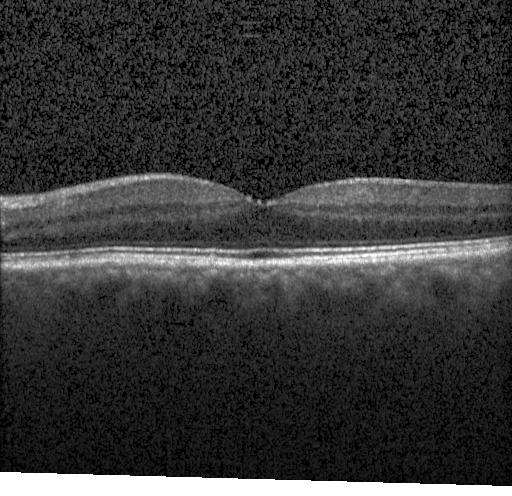 Heidelberg Spectralis; retinal OCT cross-section. Diagnosis: no evidence of CNV, DME, or drusen.